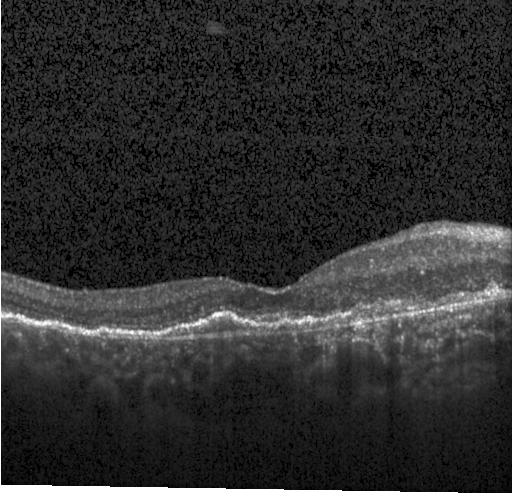
Macular scan, spectral-domain optical coherence tomography, optical coherence tomography scan.
Impression: CNV.